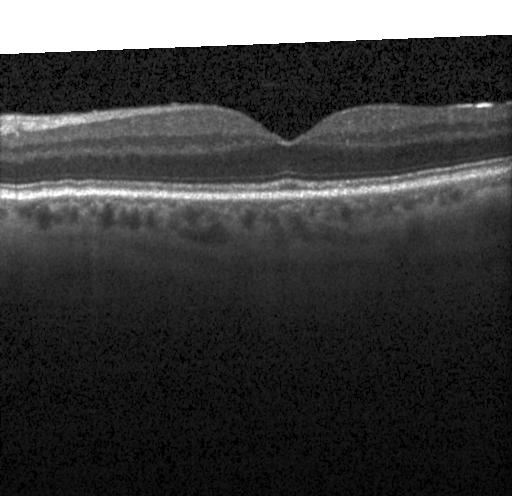
SD-OCT; through the macula; instrument: Heidelberg Spectralis; optical coherence tomography scan. This B-scan demonstrates neither CNV, DME, nor drusen.